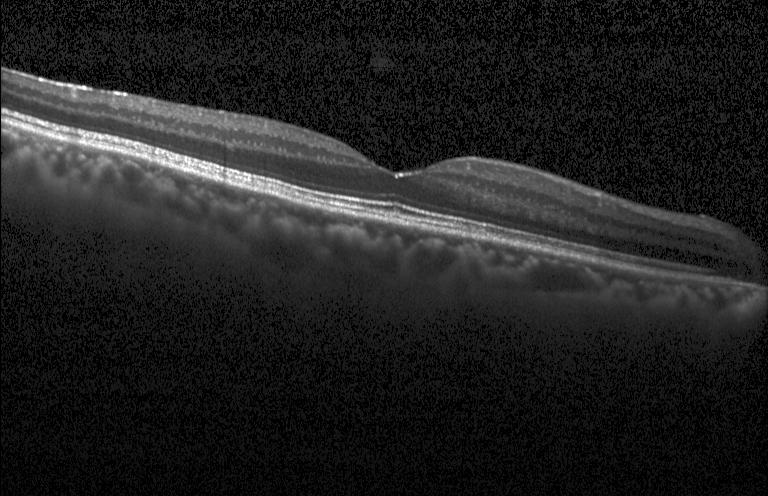
Dx: no evidence of choroidal neovascularization, diabetic macular edema, or drusen.